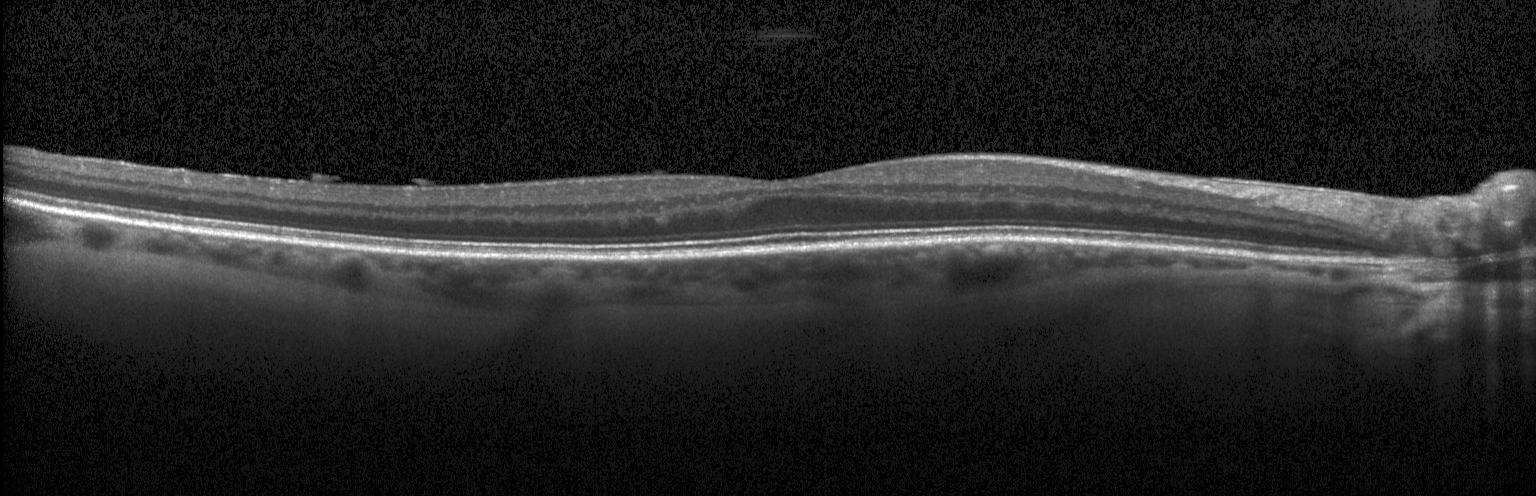

The scan shows neither choroidal neovascularization, diabetic macular edema, nor drusen.